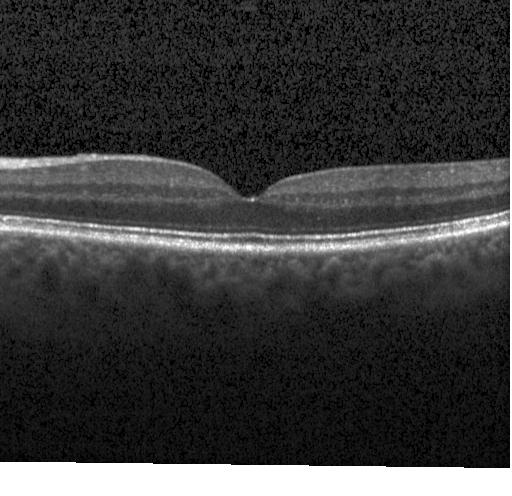
Acquired on a Heidelberg Spectralis; optical coherence tomography scan
OCT finding: no evidence of choroidal neovascularization, diabetic macular edema, or drusen.